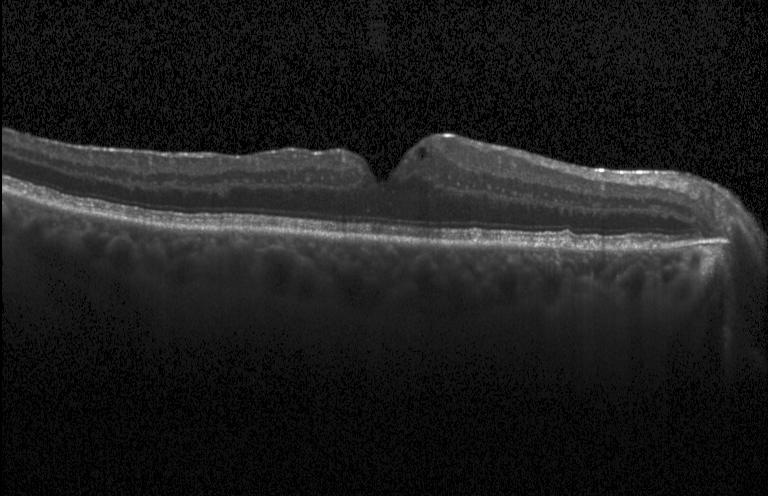

Optical coherence tomography B-scan; acquired on a Heidelberg Spectralis; spectral-domain optical coherence tomography; fovea-centered. Finding: diabetic macular edema (DME).